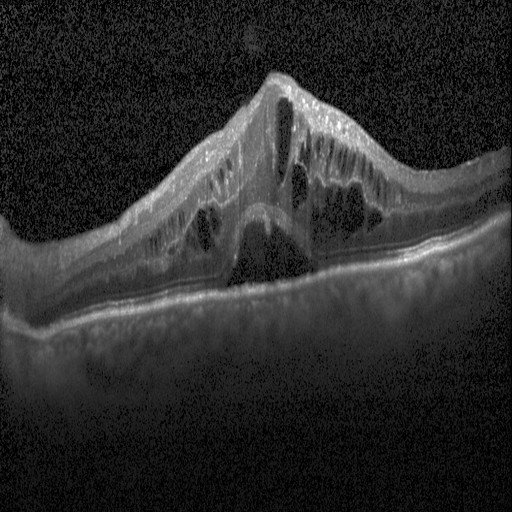 Optical coherence tomography B-scan. Finding: diabetic macular edema (DME).